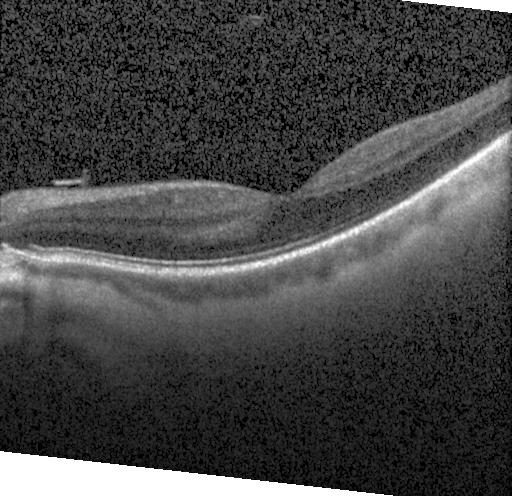

Optical coherence tomography scan — Assessment: neither CNV, DME, nor drusen.